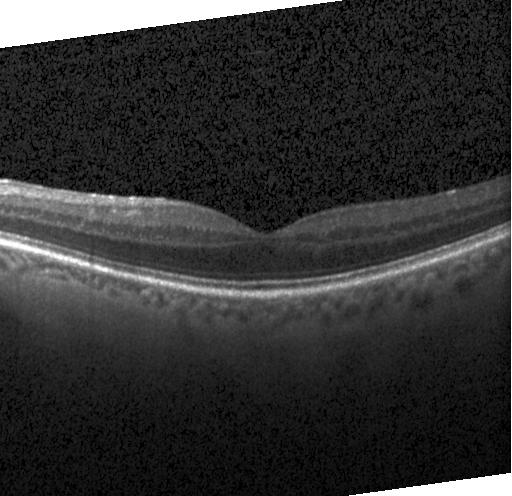
Optical coherence tomography B-scan, centered on the fovea — Impression: no choroidal neovascularization, diabetic macular edema, or drusen.